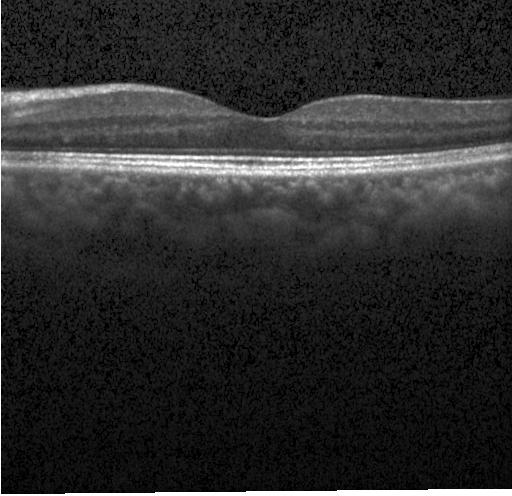
Heidelberg Spectralis · spectral-domain optical coherence tomography · retinal OCT B-scan · through the macula.
Impression: no evidence of choroidal neovascularization, diabetic macular edema, or drusen.